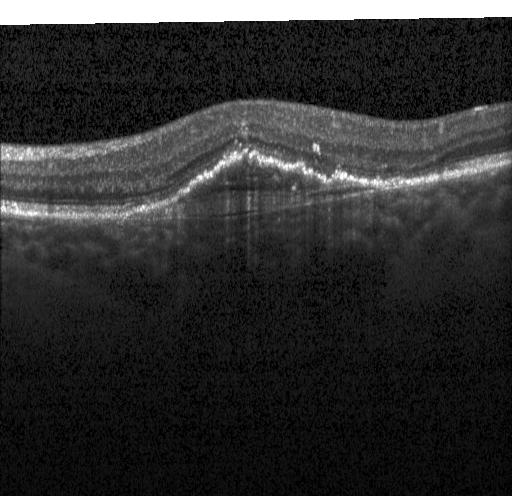

Instrument: Heidelberg Spectralis. OCT line scan — This B-scan demonstrates a choroidal neovascular membrane.